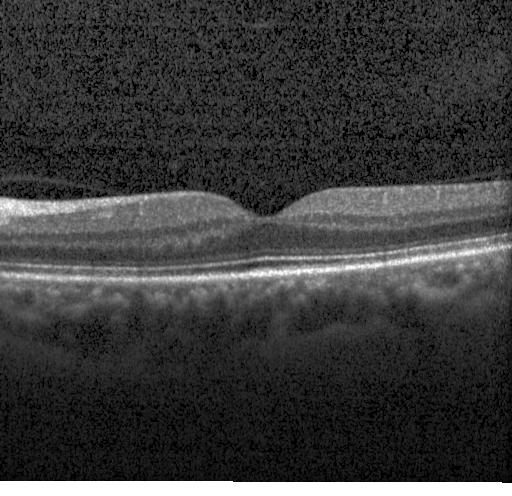

Acquired on a Heidelberg Spectralis; optical coherence tomography scan.
Assessment: no choroidal neovascularization, diabetic macular edema, or drusen.